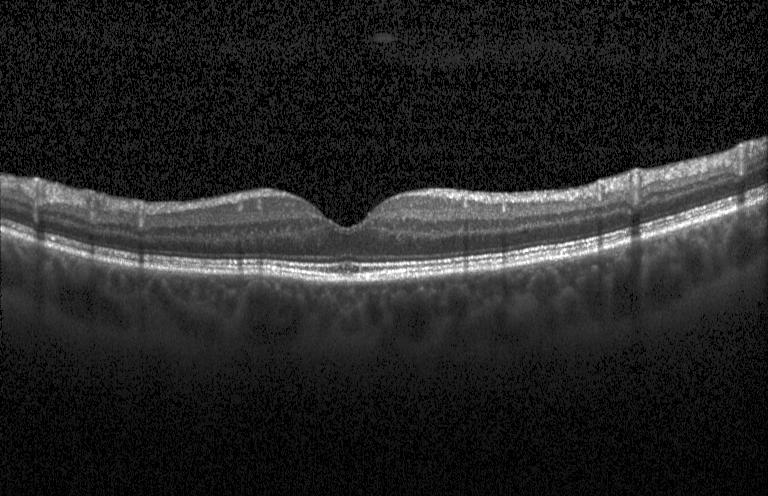 Finding: no evidence of CNV, DME, or drusen.